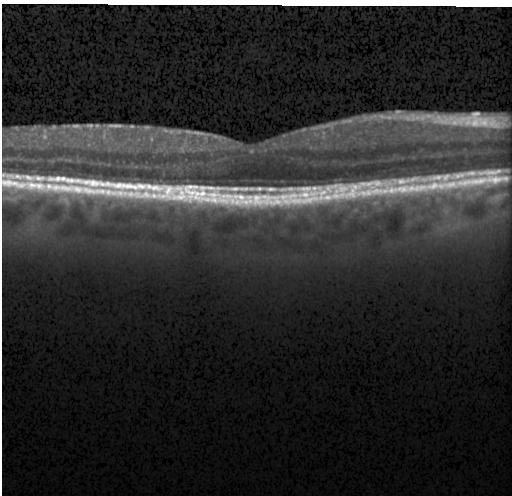

Optical coherence tomography B-scan
This B-scan demonstrates no evidence of choroidal neovascularization, diabetic macular edema, or drusen.